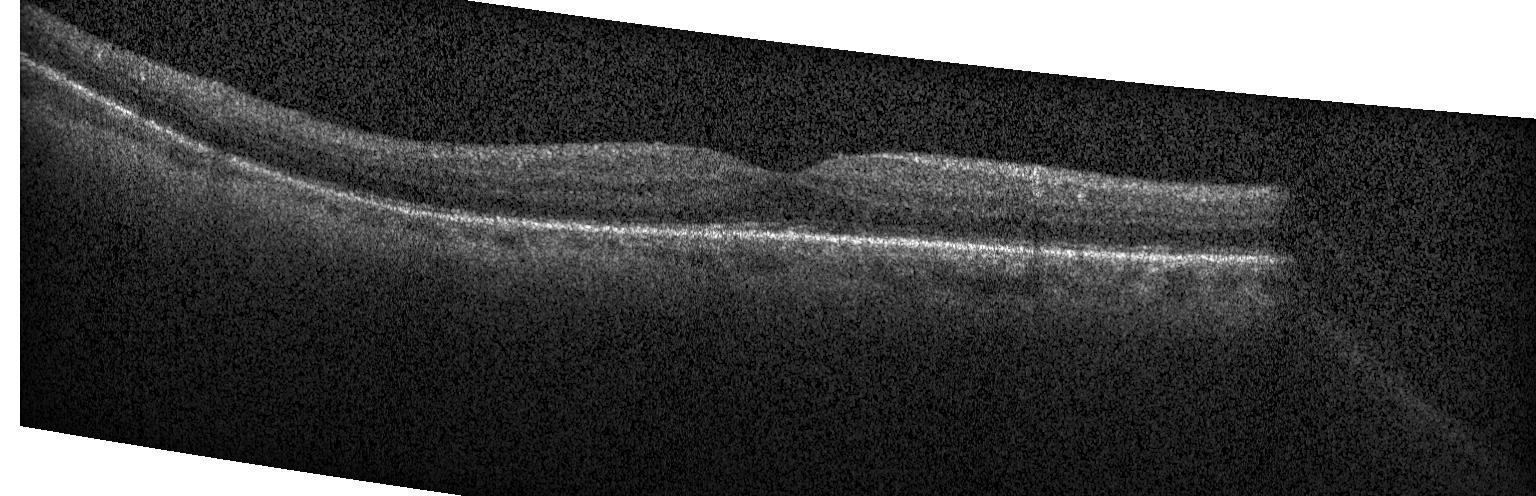

This B-scan demonstrates no CNV, no DME, and no drusen.